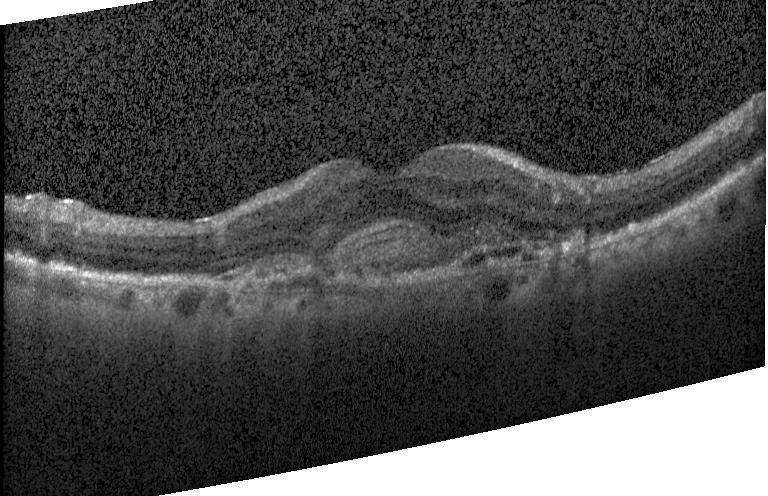 Horizontal scan through the fovea. Instrument: Heidelberg Spectralis. Spectral-domain optical coherence tomography. Optical coherence tomography scan
Diagnosis: a choroidal neovascular membrane.